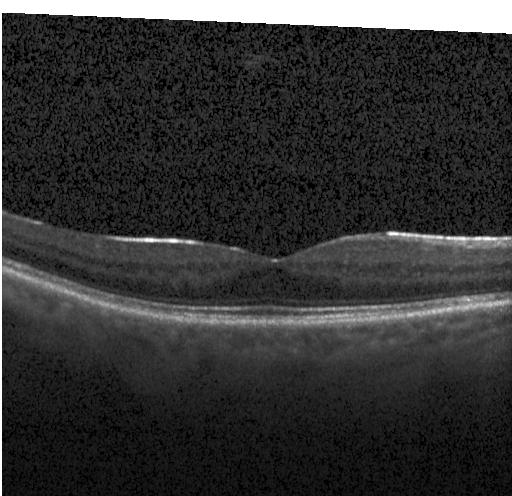

Impression: neither choroidal neovascularization, diabetic macular edema, nor drusen.